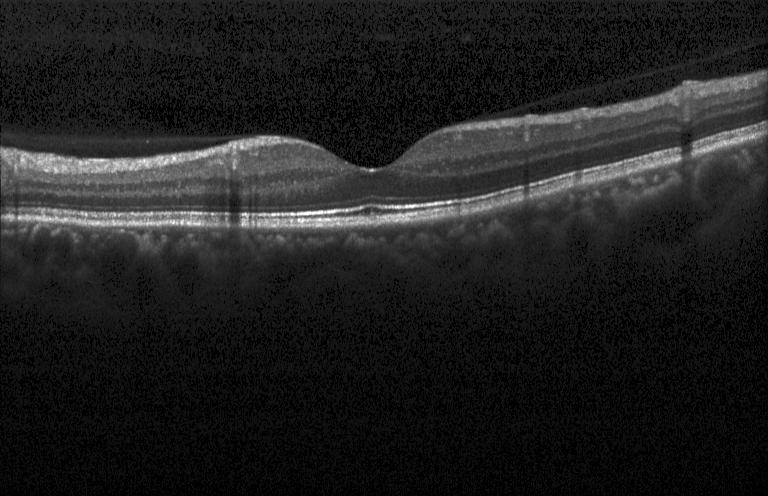 Optical coherence tomography B-scan. The scan shows no choroidal neovascularization, no diabetic macular edema, and no drusen.